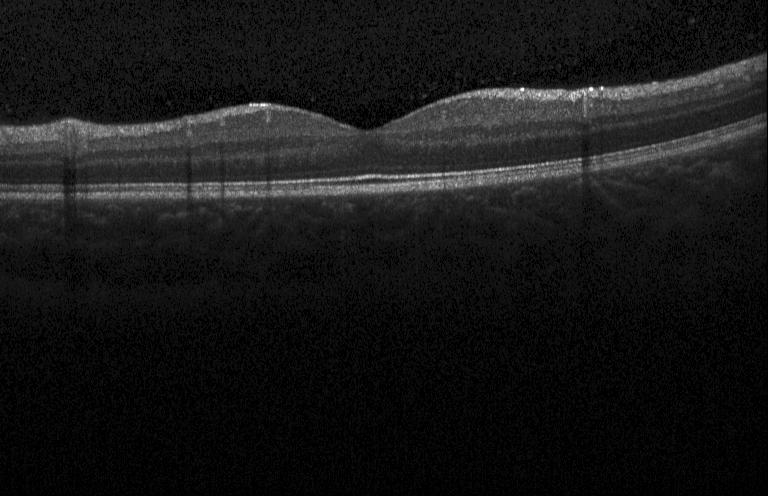
Spectral-domain optical coherence tomography, instrument: Heidelberg Spectralis, optical coherence tomography B-scan, fovea-centered.
Diagnosis: no evidence of choroidal neovascularization, diabetic macular edema, or drusen.